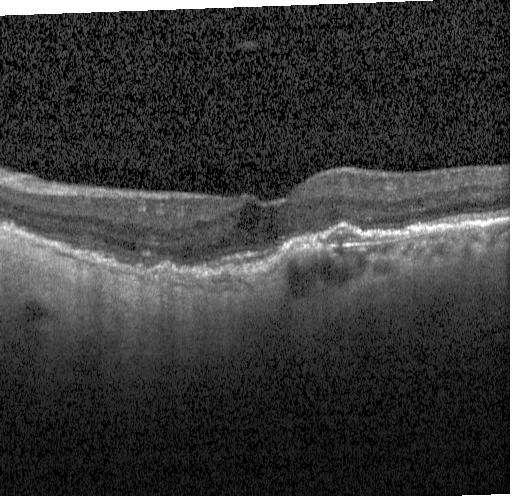 Retinal OCT B-scan. Acquired on a Heidelberg Spectralis. Horizontal scan through the fovea. Spectral-domain OCT. Diagnosis: a choroidal neovascular membrane.